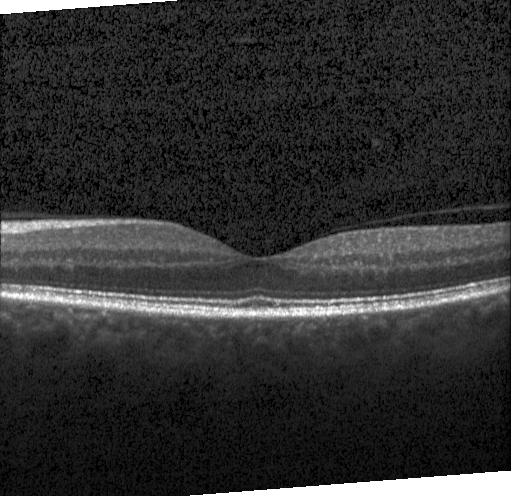

Macular scan; OCT B-scan
Dx: no choroidal neovascularization, no diabetic macular edema, and no drusen.